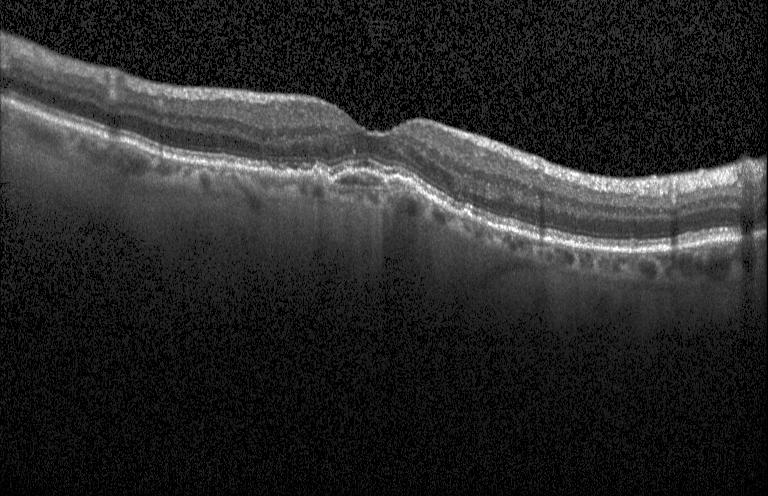 OCT B-scan showing a choroidal neovascular membrane.